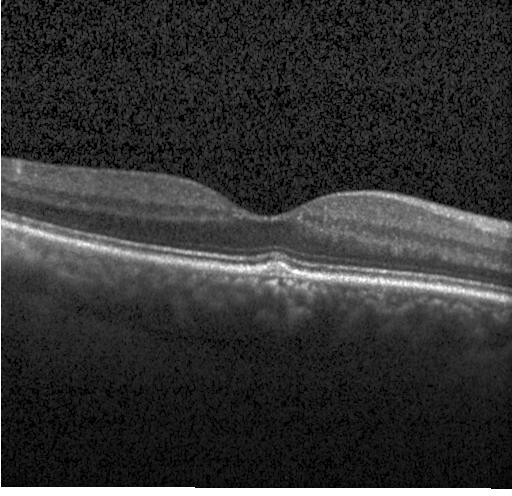

Through the macula, OCT line scan
OCT finding: multiple drusen.